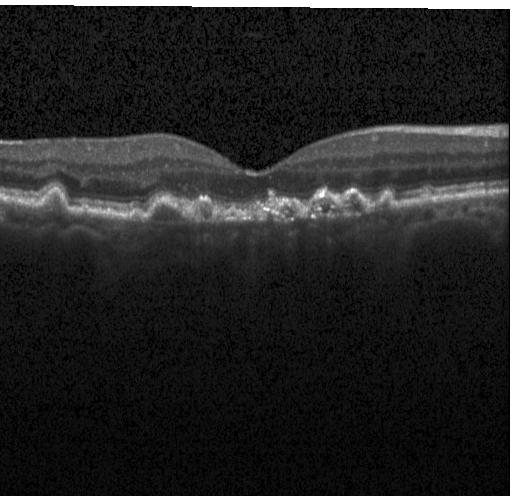
Finding: choroidal neovascularization.